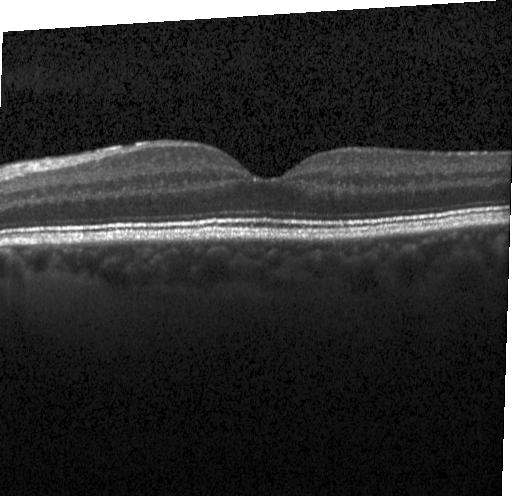 SD-OCT; OCT B-scan.
Diagnosis: no choroidal neovascularization, no diabetic macular edema, and no drusen.